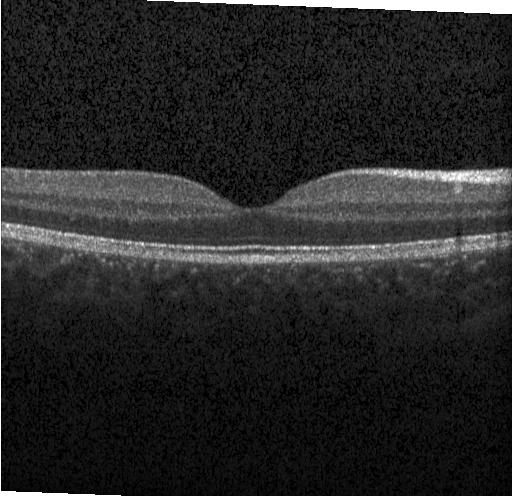 Spectral-domain OCT; optical coherence tomography scan; centered on the fovea; acquired on a Heidelberg Spectralis
Impression: no evidence of choroidal neovascularization, diabetic macular edema, or drusen.